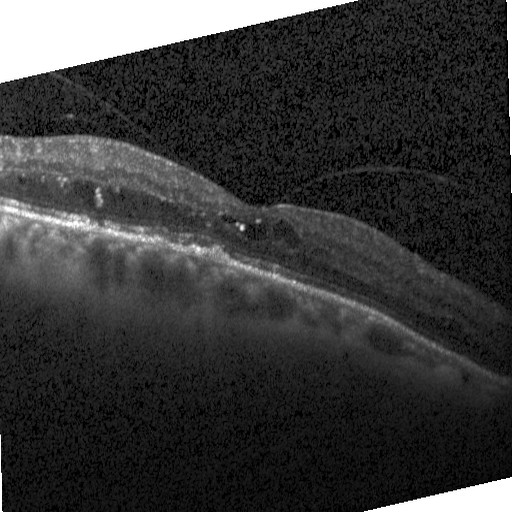

Optical coherence tomography scan, spectral-domain OCT.
Finding: diabetic macular edema.